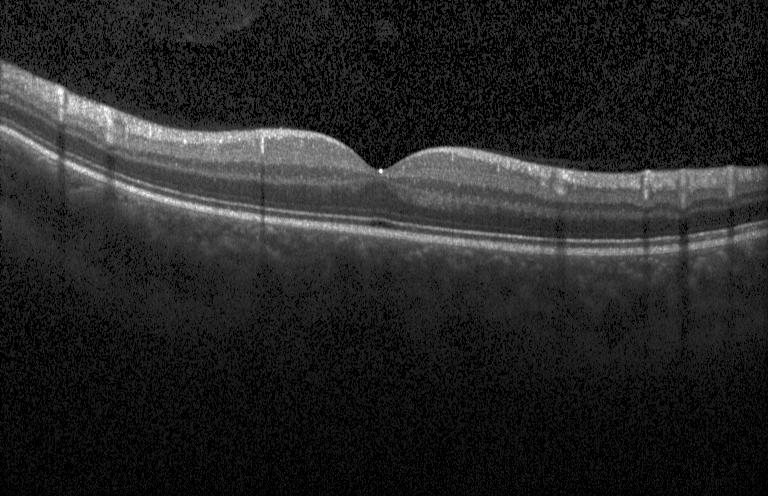
Optical coherence tomography scan.
Assessment: neither choroidal neovascularization, diabetic macular edema, nor drusen.